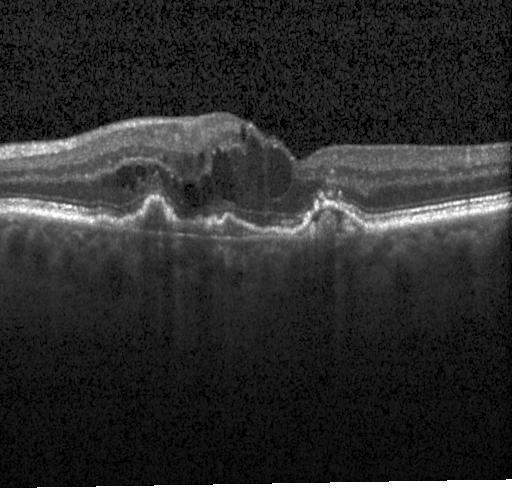

Spectral-domain OCT; OCT B-scan; horizontal scan through the fovea. Diagnosis: a choroidal neovascular membrane.